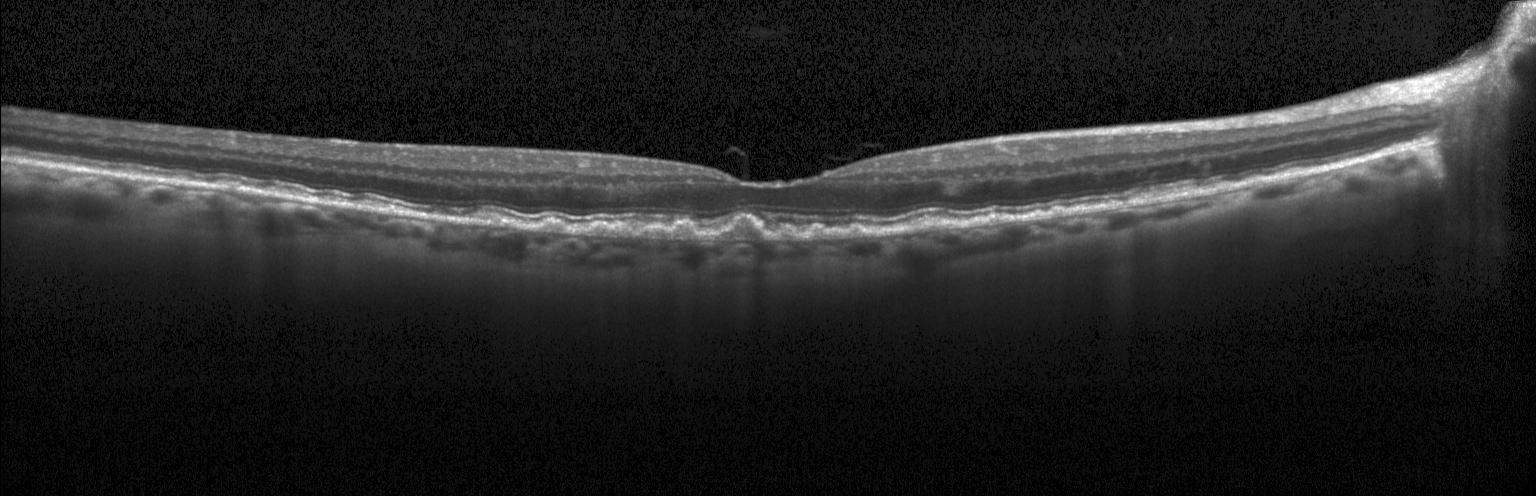 OCT line scan. Spectral-domain OCT
Macular OCT: drusen.